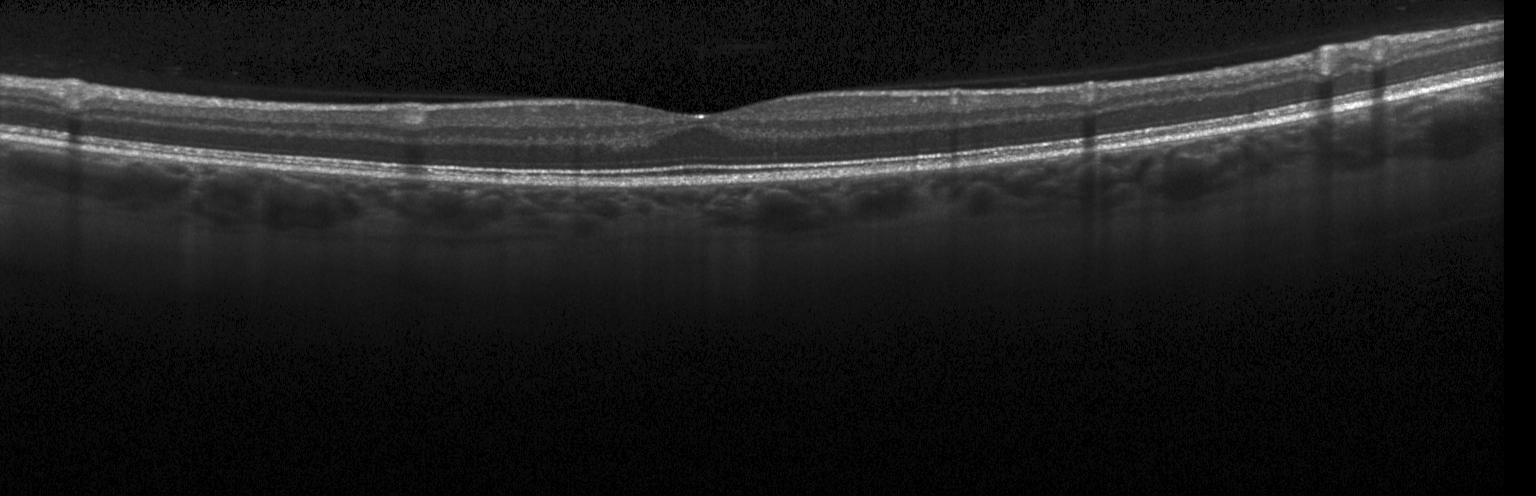

No evidence of choroidal neovascularization, diabetic macular edema, or drusen.